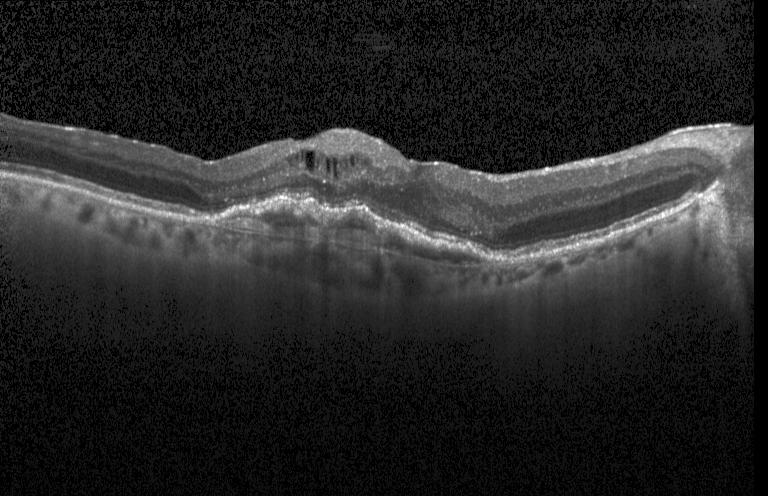

Instrument: Heidelberg Spectralis; retinal OCT B-scan — OCT finding: a choroidal neovascular membrane.